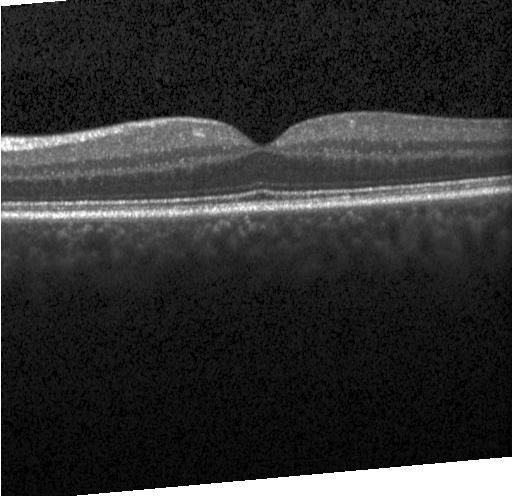 Macular OCT: neither choroidal neovascularization, diabetic macular edema, nor drusen.